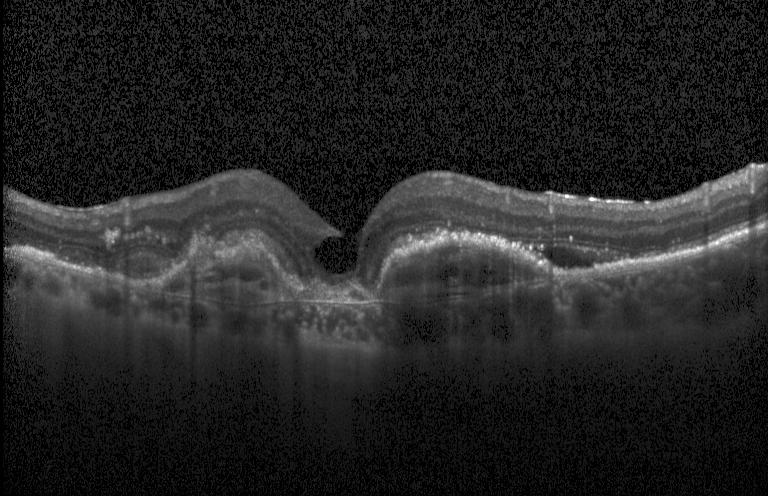

Macular scan; spectral-domain OCT; Heidelberg Spectralis OCT system; retinal OCT cross-section.
This B-scan demonstrates a choroidal neovascular membrane.